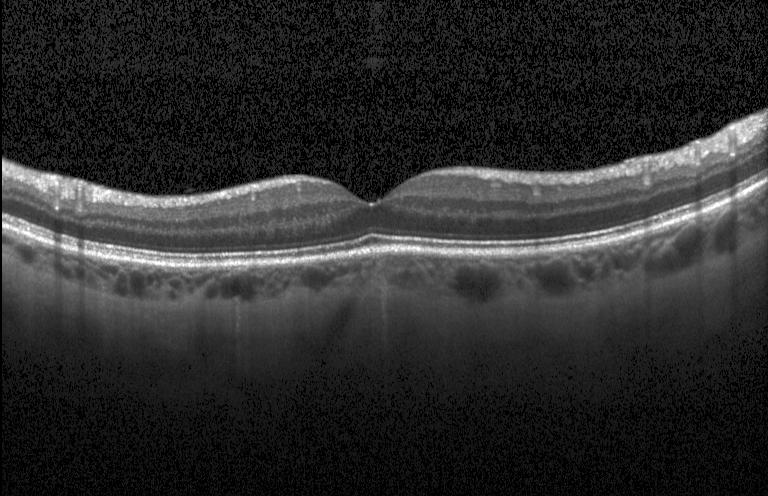
OCT B-scan showing neither choroidal neovascularization, diabetic macular edema, nor drusen.